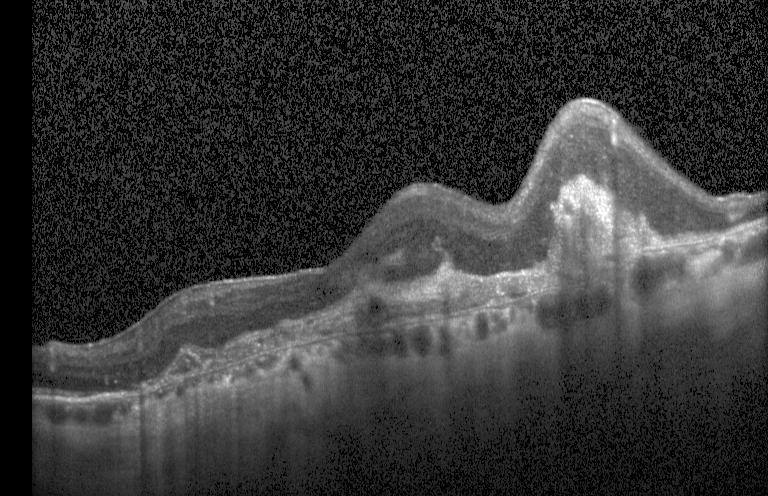
Macular OCT: choroidal neovascularization (CNV).